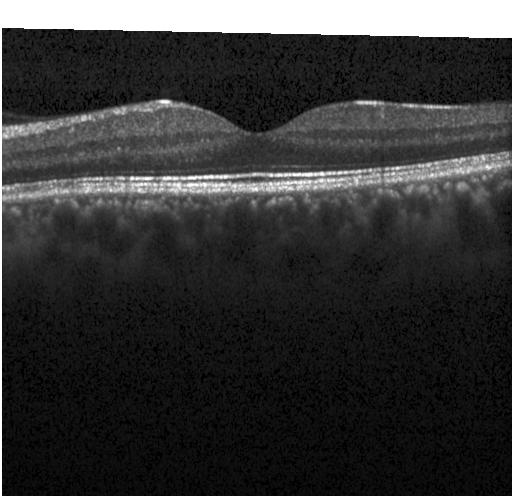 Macular OCT demonstrating no choroidal neovascularization, diabetic macular edema, or drusen.